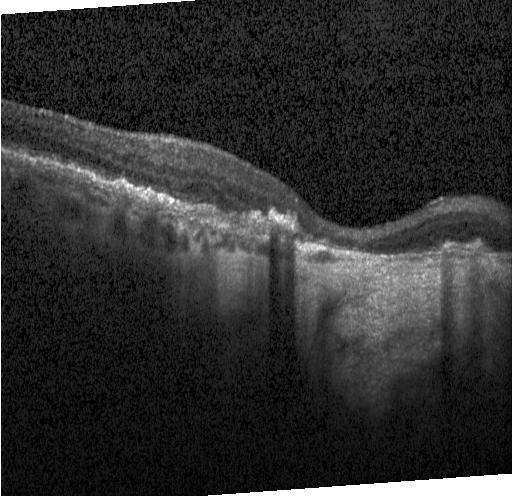
Diagnosis: a choroidal neovascular membrane.